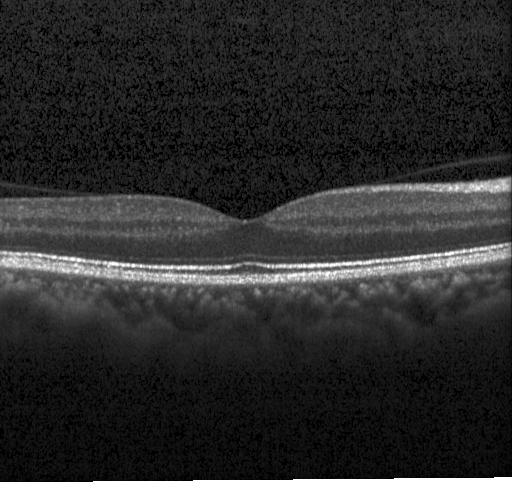 Optical coherence tomography scan · SD-OCT — No choroidal neovascularization, diabetic macular edema, or drusen.